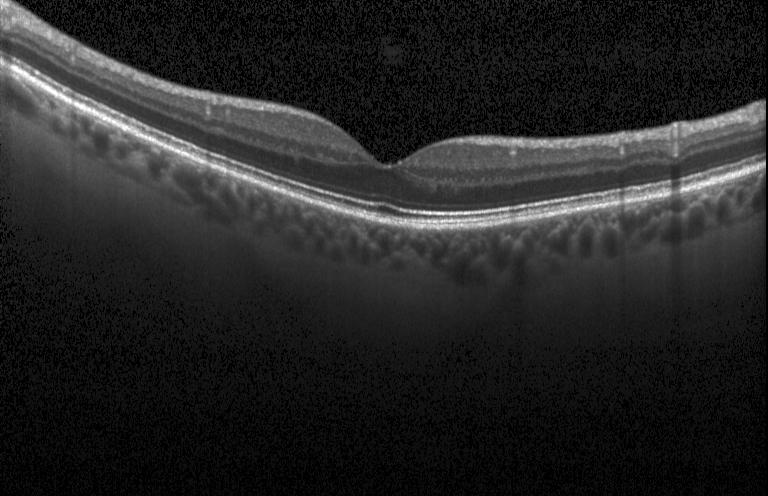 Acquired on a Heidelberg Spectralis · retinal OCT cross-section. OCT finding: no choroidal neovascularization, diabetic macular edema, or drusen.